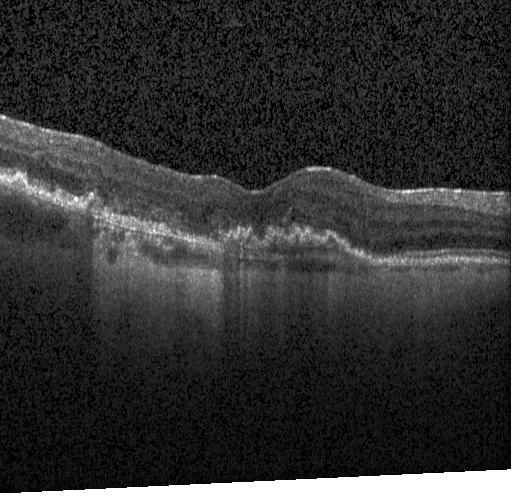
Instrument: Heidelberg Spectralis · spectral-domain OCT · fovea-centered · optical coherence tomography scan.
Macular OCT: a choroidal neovascular membrane.